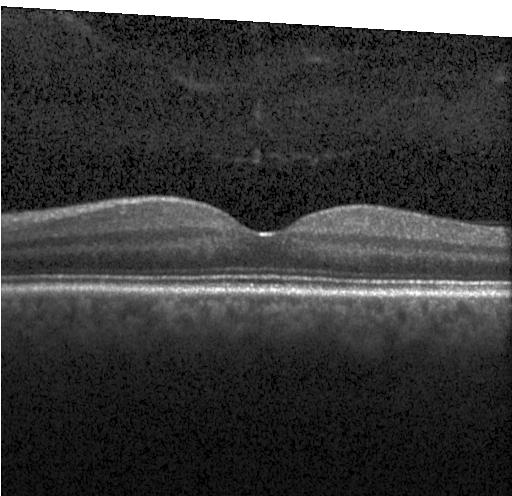 Optical coherence tomography B-scan
The scan shows no choroidal neovascularization, no diabetic macular edema, and no drusen.